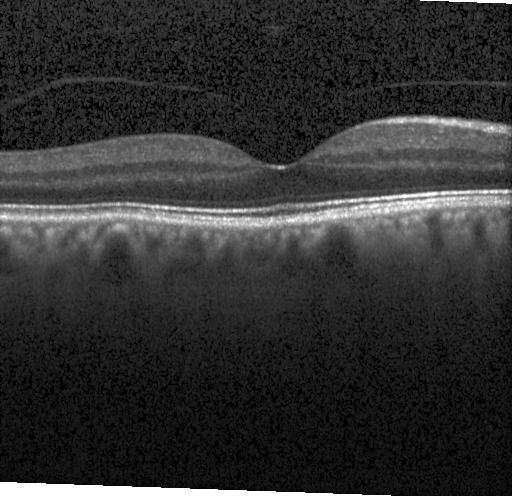

OCT line scan. SD-OCT. Instrument: Heidelberg Spectralis. Fovea-centered — Diagnosis: no CNV, DME, or drusen.